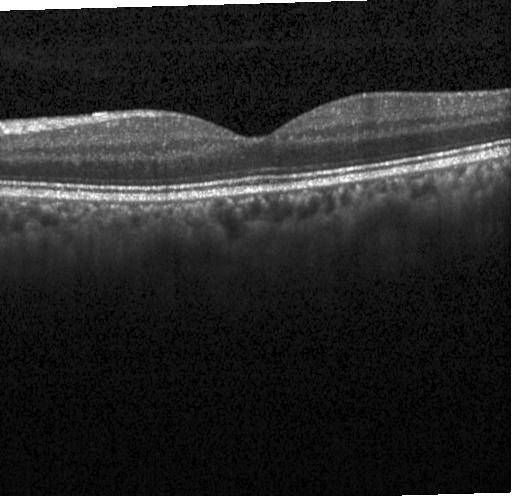

OCT line scan.
Dx: no evidence of choroidal neovascularization, diabetic macular edema, or drusen.